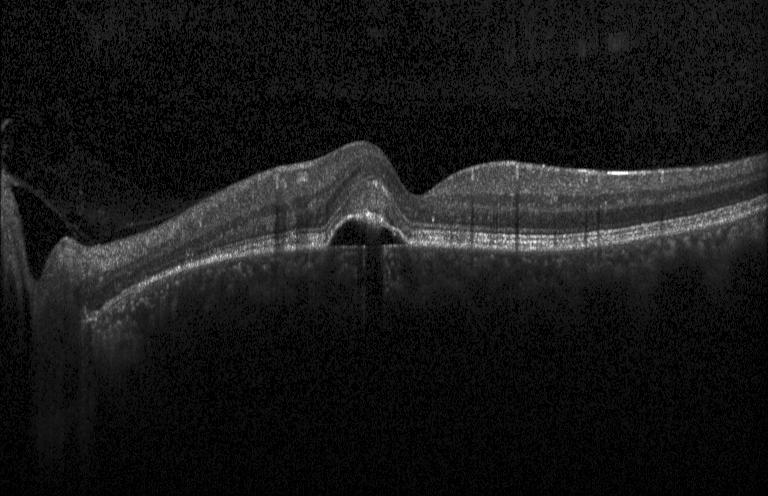

Impression: a choroidal neovascular membrane.